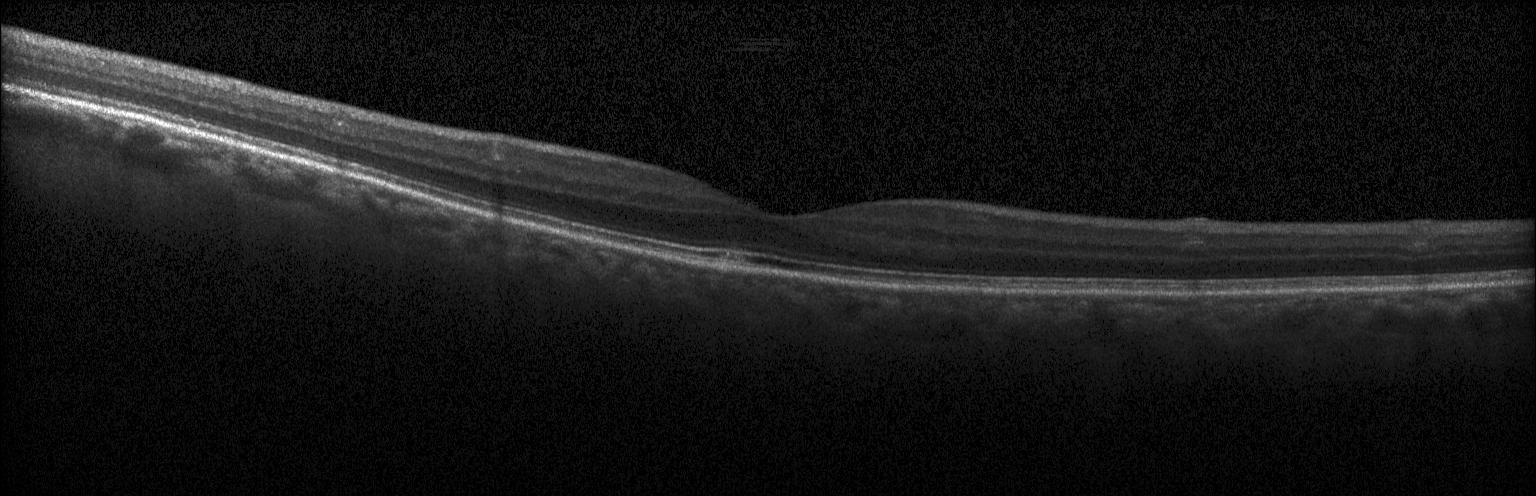

The scan shows no choroidal neovascularization, no diabetic macular edema, and no drusen.